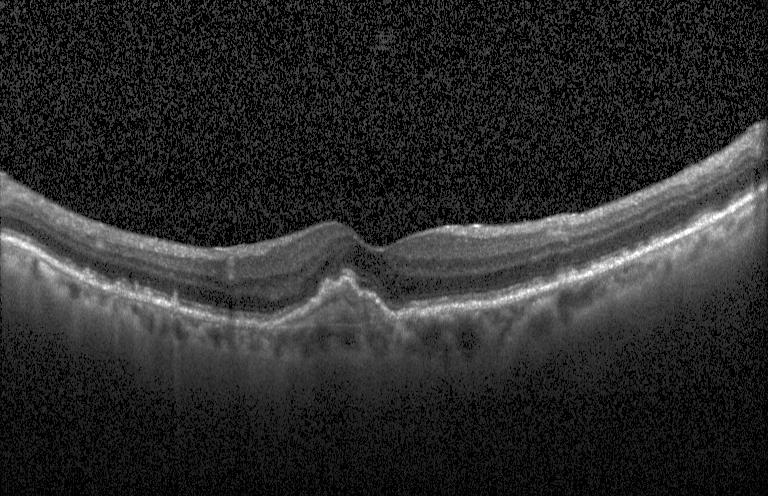

Spectral-domain OCT B-scan: choroidal neovascularization (CNV).